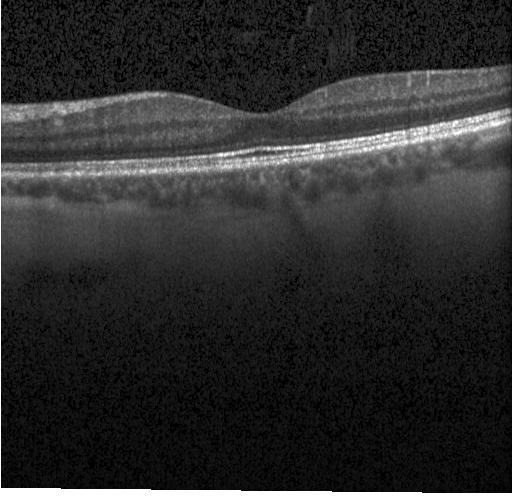 Retinal OCT cross-section · fovea-centered · SD-OCT · acquired on a Heidelberg Spectralis. Diagnosis: no evidence of choroidal neovascularization, diabetic macular edema, or drusen.